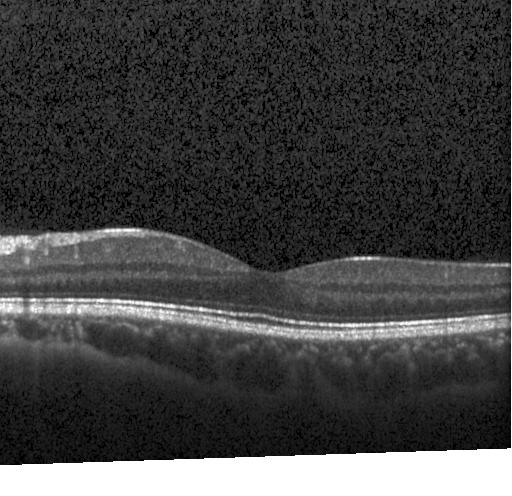 Macular OCT: neither choroidal neovascularization, diabetic macular edema, nor drusen.